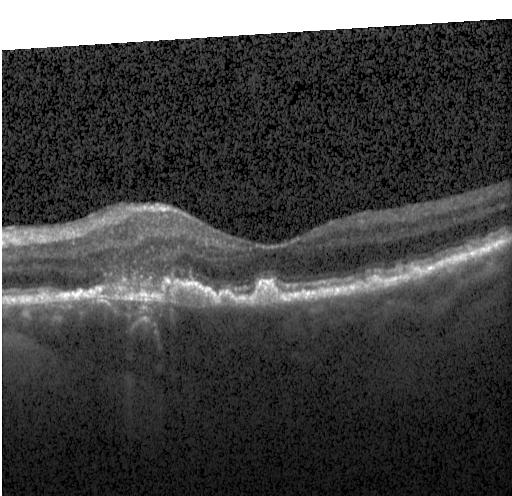 Retinal OCT cross-section; spectral-domain OCT.
Finding: a choroidal neovascular membrane.